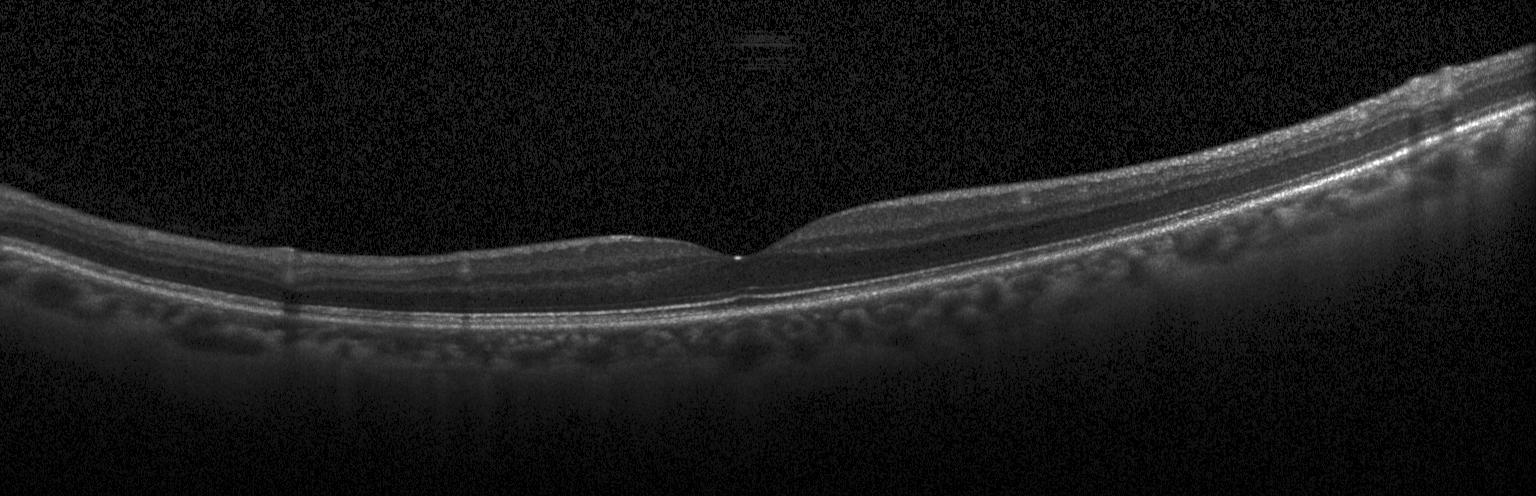 No choroidal neovascularization, diabetic macular edema, or drusen.